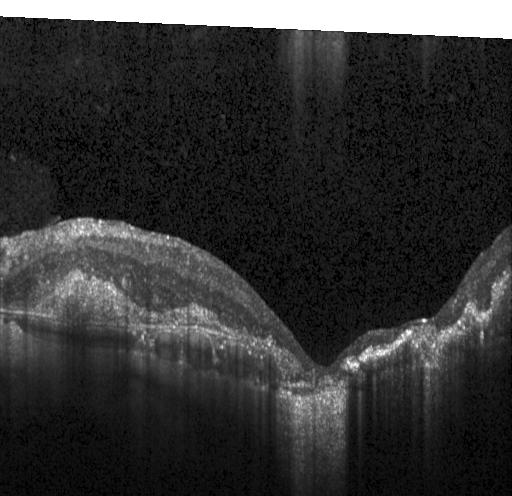 SD-OCT. OCT line scan. Assessment: CNV.